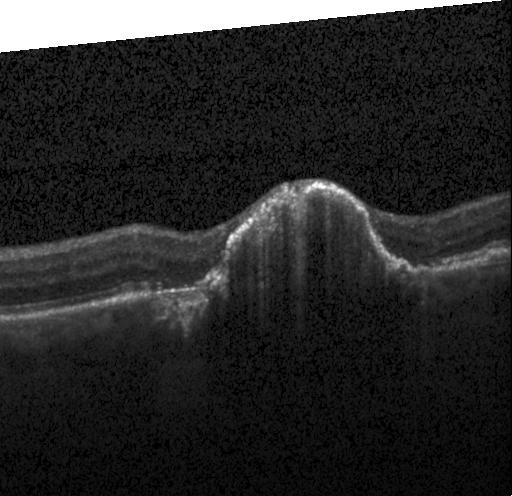 Through the macula · OCT B-scan. This B-scan demonstrates a choroidal neovascular membrane.